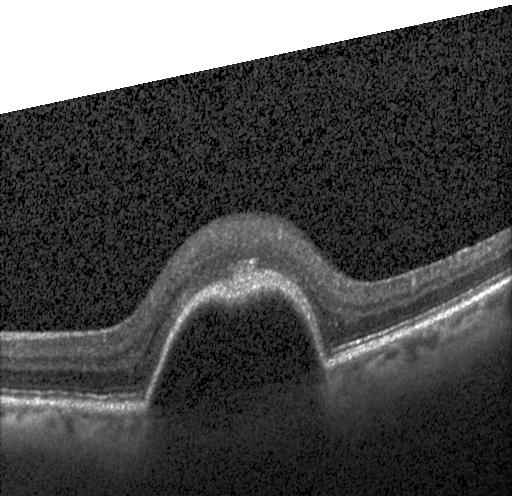

The scan shows a choroidal neovascular membrane.